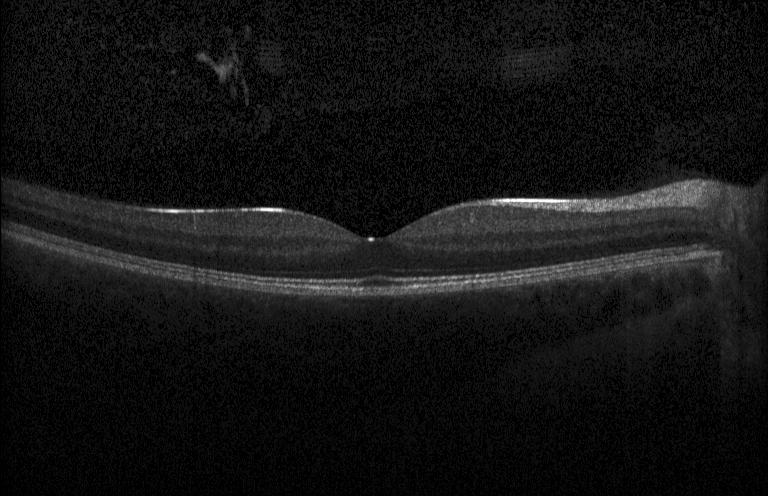
OCT B-scan. No choroidal neovascularization, diabetic macular edema, or drusen.